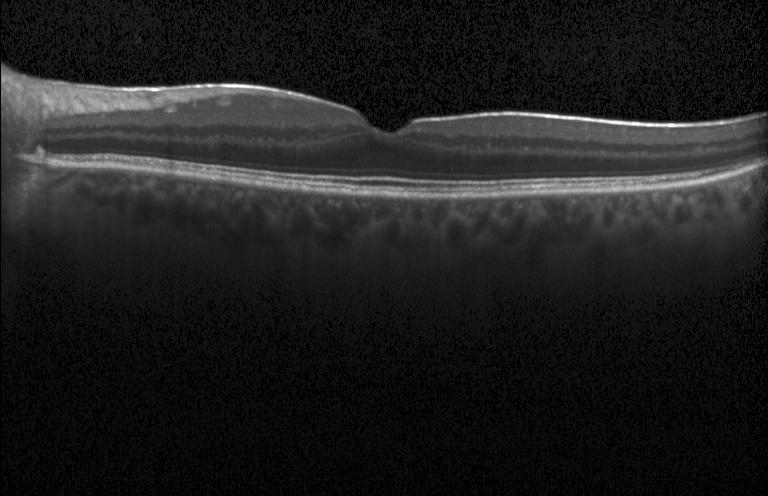

Retinal OCT B-scan; spectral-domain optical coherence tomography; Heidelberg Spectralis; horizontal scan through the fovea. Assessment: no choroidal neovascularization, diabetic macular edema, or drusen.